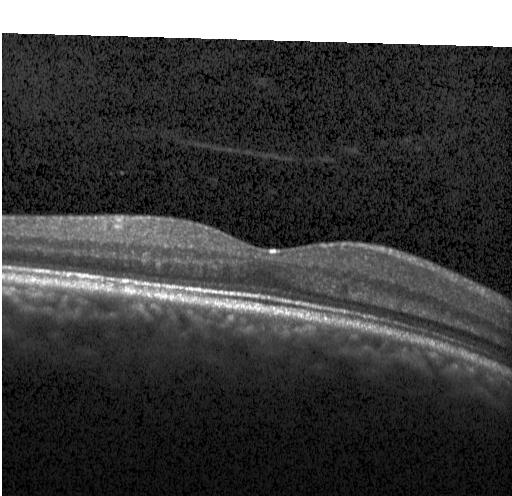
OCT line scan, spectral-domain OCT — Assessment: no evidence of CNV, DME, or drusen.